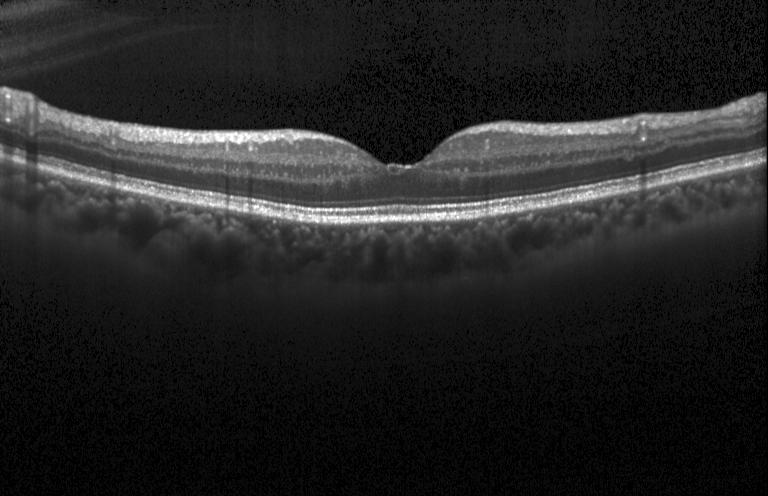 Centered on the fovea, acquired on a Heidelberg Spectralis, optical coherence tomography B-scan, spectral-domain OCT. Impression: no choroidal neovascularization, diabetic macular edema, or drusen.